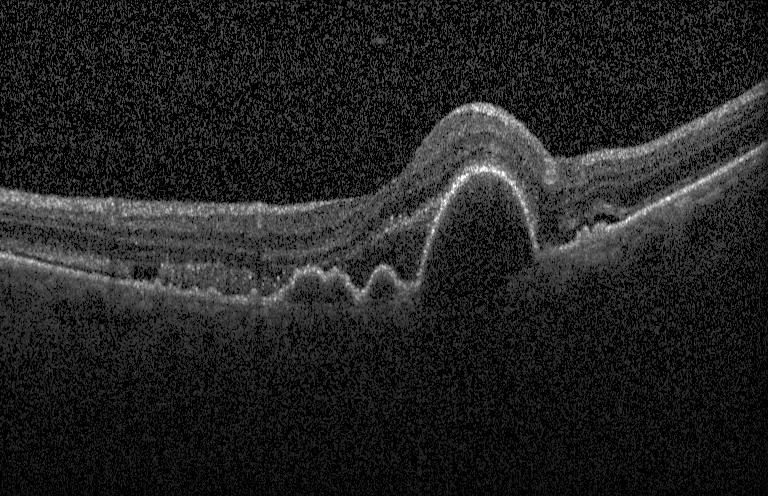 Optical coherence tomography B-scan
The scan shows choroidal neovascularization (CNV).